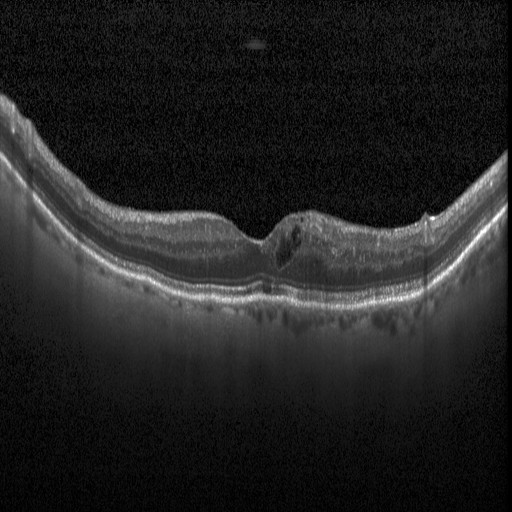 Finding: DME.